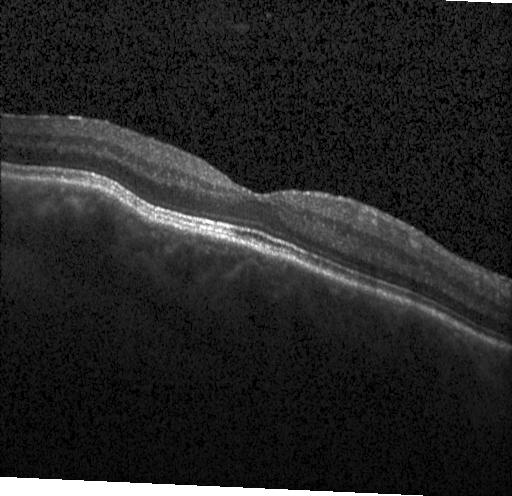
OCT line scan.
Impression: no evidence of choroidal neovascularization, diabetic macular edema, or drusen.